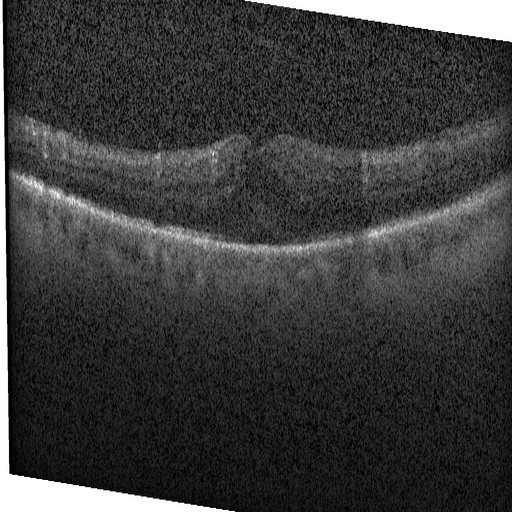
This B-scan demonstrates diabetic macular edema.